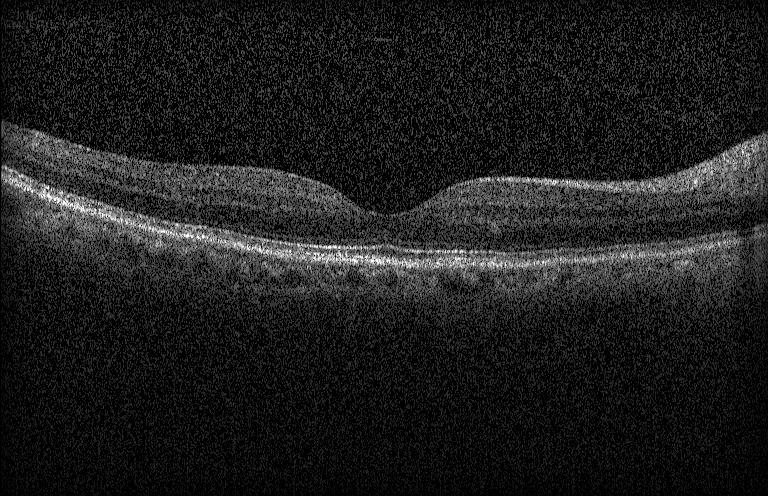
Macular scan. Retinal OCT cross-section. Spectral-domain OCT.
Finding: no choroidal neovascularization, diabetic macular edema, or drusen.